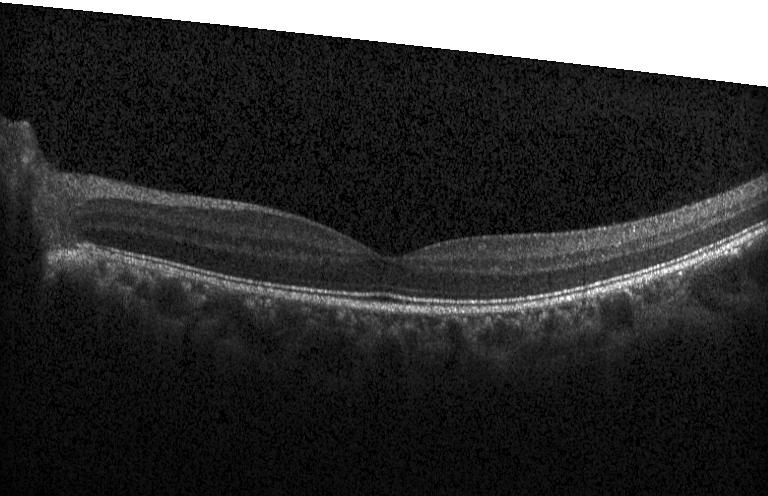 OCT line scan, instrument: Heidelberg Spectralis. OCT finding: no choroidal neovascularization, no diabetic macular edema, and no drusen.